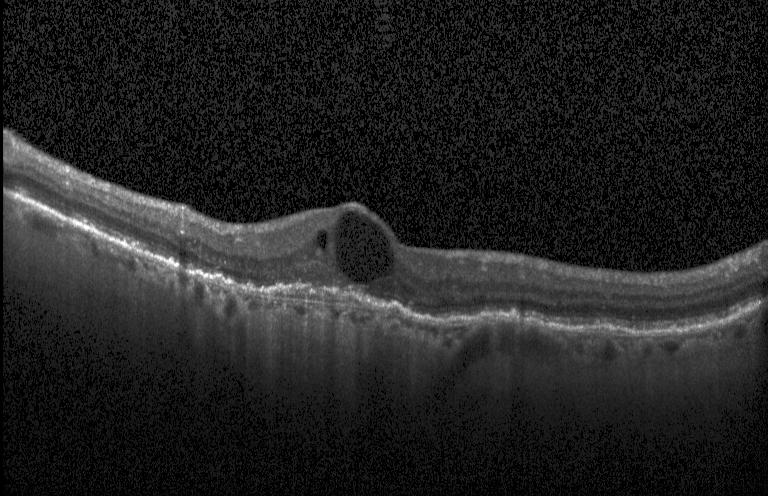

SD-OCT, OCT line scan, acquired on a Heidelberg Spectralis
The scan shows choroidal neovascularization (CNV).